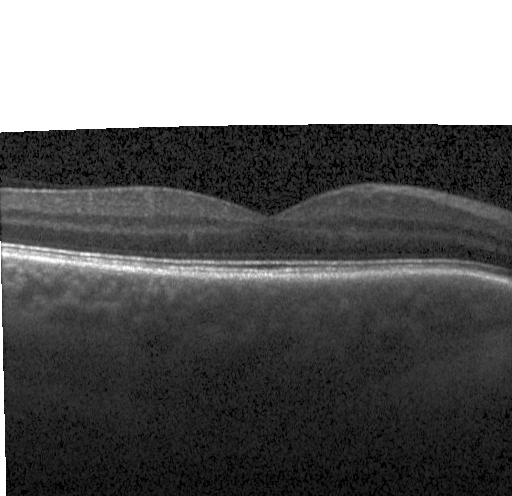

Finding: no CNV, DME, or drusen.